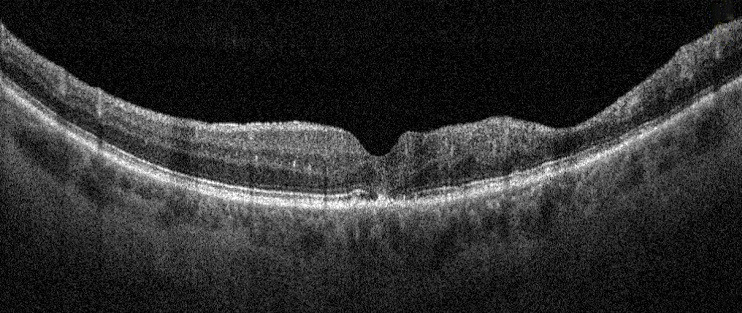 Dx: RVO.